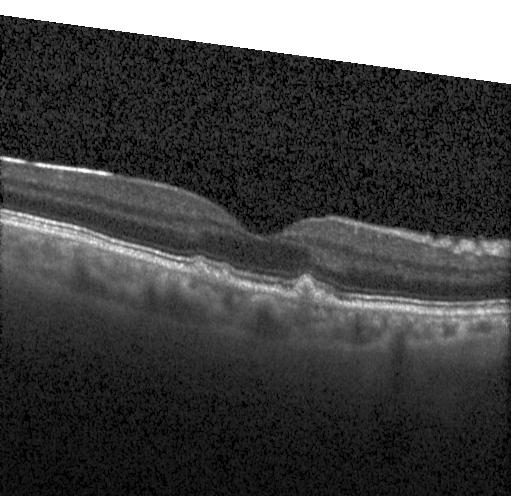 OCT B-scan — This B-scan demonstrates sub-RPE drusenoid deposits.